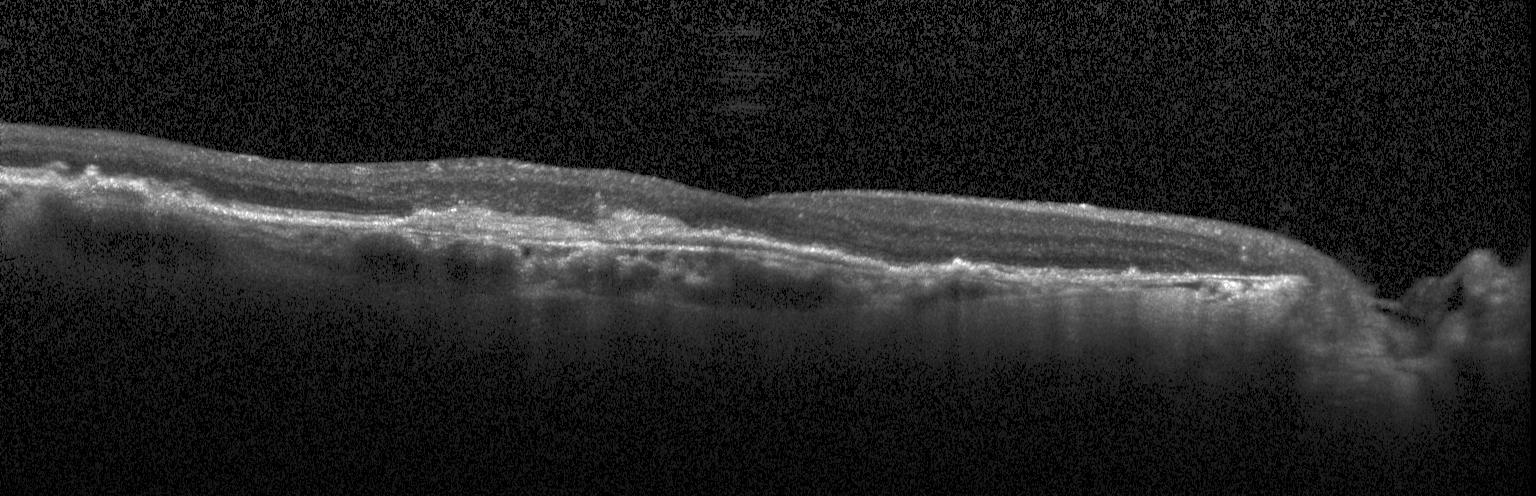 Optical coherence tomography B-scan
Diagnosis: a choroidal neovascular membrane.